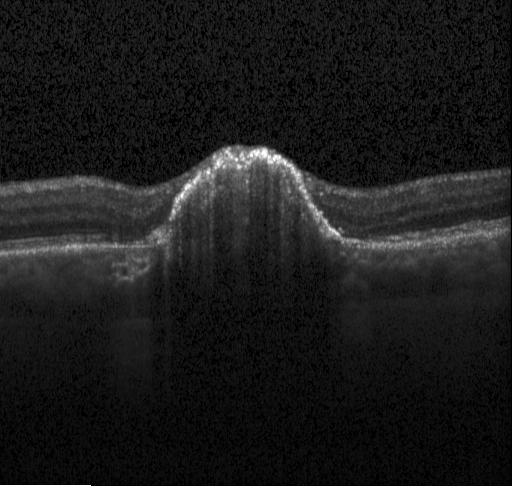 Retinal OCT B-scan. OCT finding: a choroidal neovascular membrane.